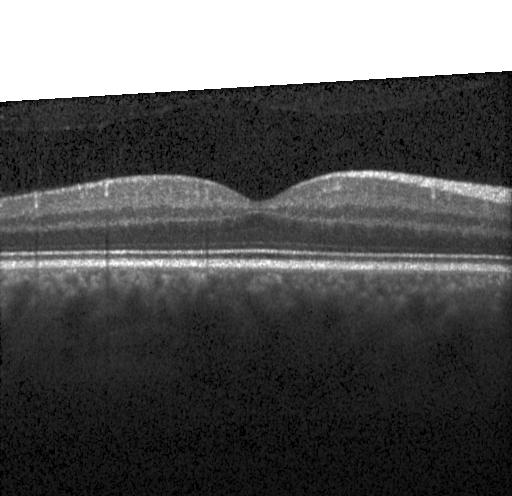 Spectral-domain OCT · OCT B-scan · macular scan. The scan shows no evidence of choroidal neovascularization, diabetic macular edema, or drusen.